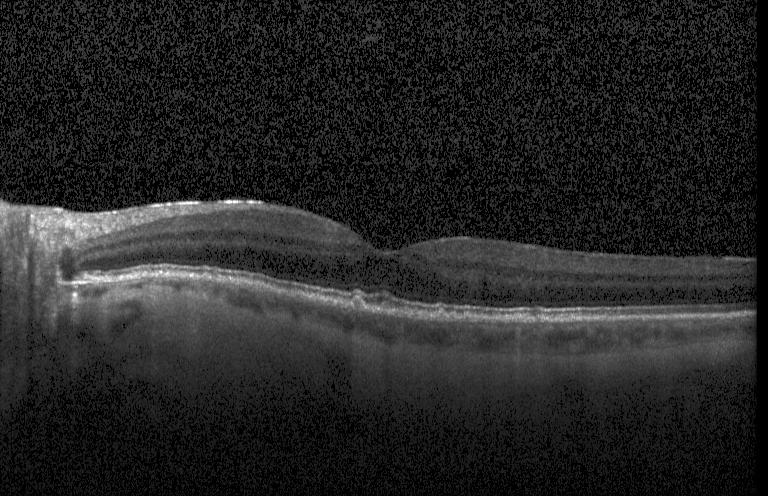
Spectral-domain optical coherence tomography, Heidelberg Spectralis, OCT line scan
This B-scan demonstrates sub-RPE drusenoid deposits.